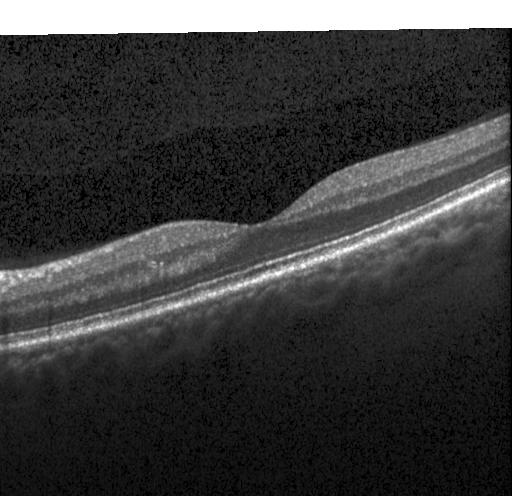

Macular scan · instrument: Heidelberg Spectralis · optical coherence tomography B-scan.
Diagnosis: no choroidal neovascularization, no diabetic macular edema, and no drusen.